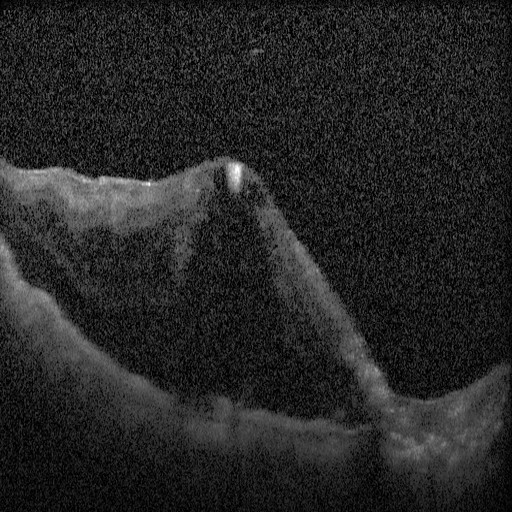
Retinal OCT cross-section
Finding: diabetic macular edema.